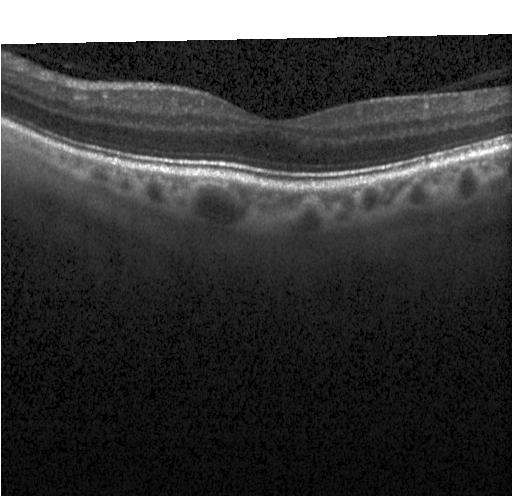
OCT scan showing no evidence of choroidal neovascularization, diabetic macular edema, or drusen.